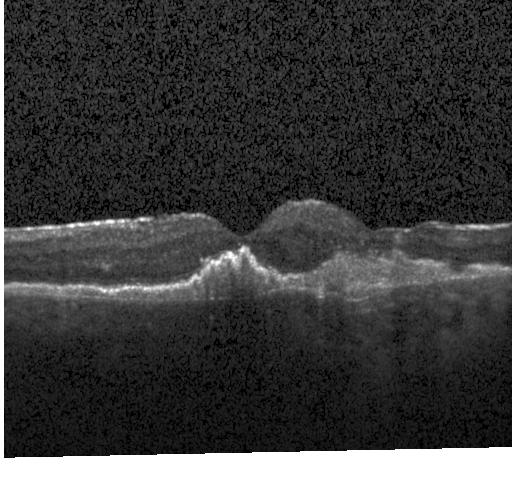 OCT line scan — Dx: CNV.